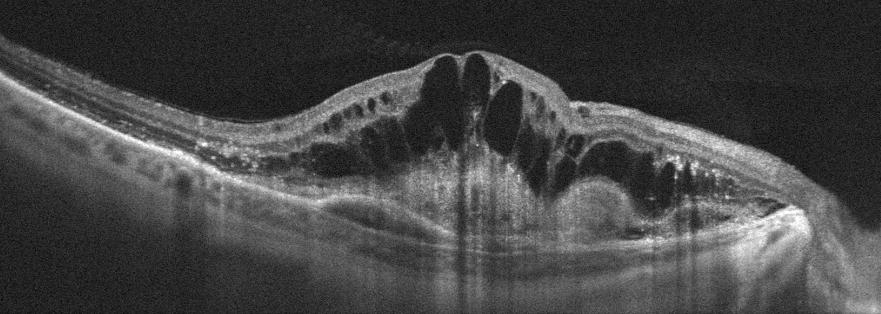 Retinal OCT B-scan. Diagnosis: age-related macular degeneration (AMD).